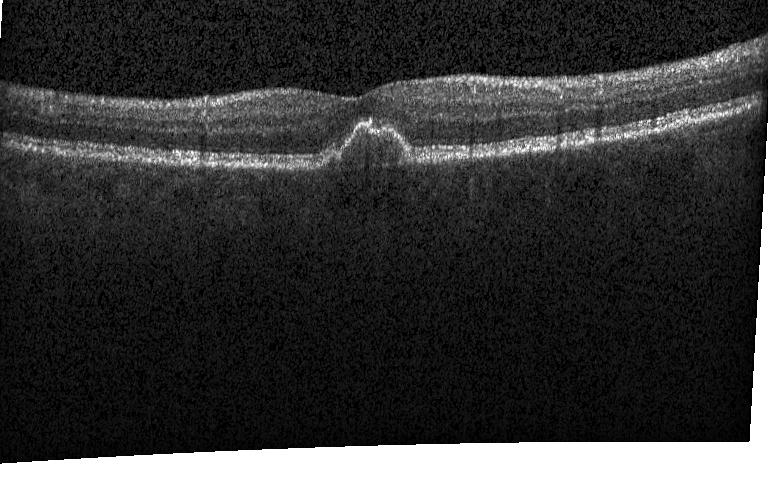

Impression: multiple drusen.